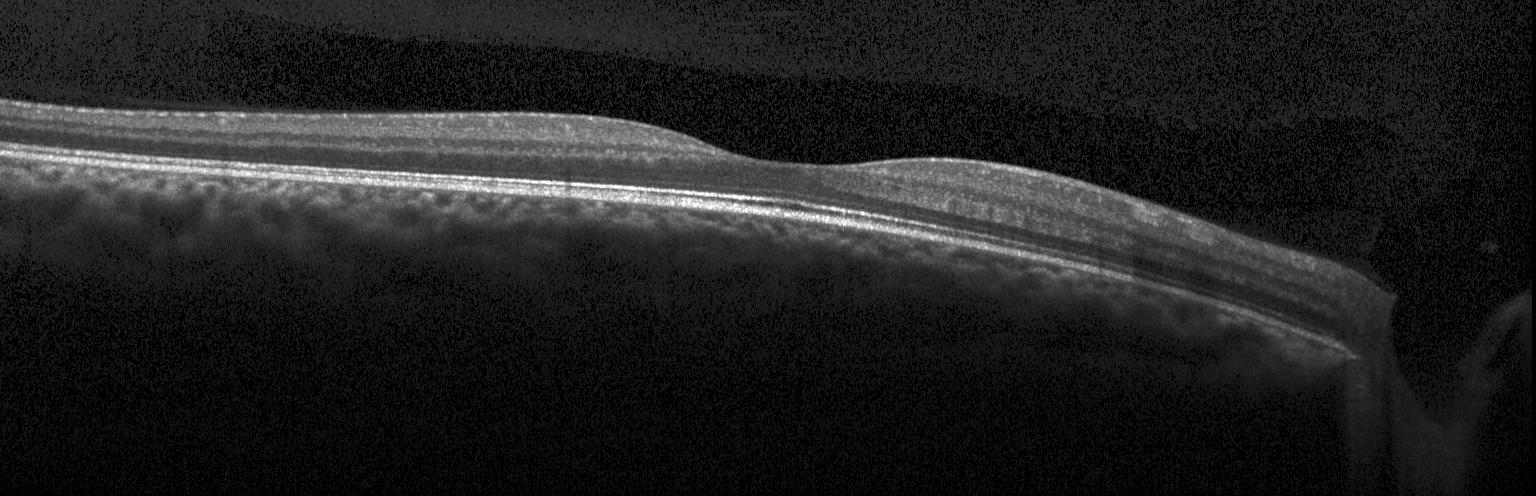 OCT line scan — Finding: no choroidal neovascularization, diabetic macular edema, or drusen.